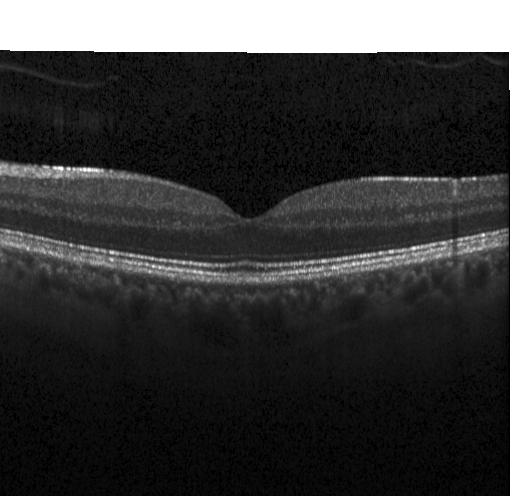 Macular OCT: no CNV, DME, or drusen.